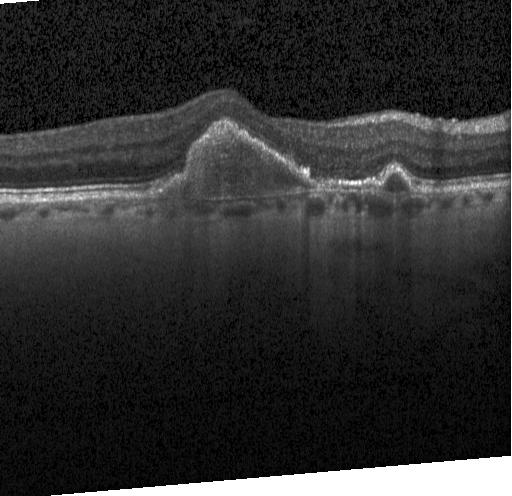
Retinal OCT B-scan; spectral-domain optical coherence tomography; macular scan; Heidelberg Spectralis OCT system.
The scan shows choroidal neovascularization (CNV).